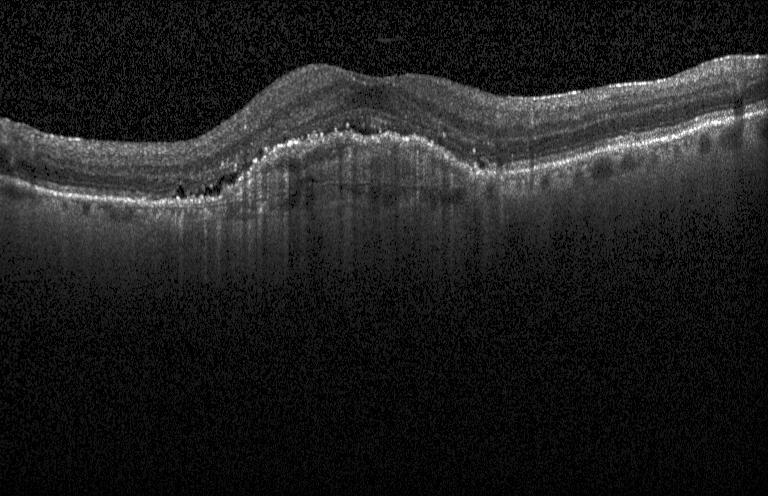
Choroidal neovascularization (CNV).